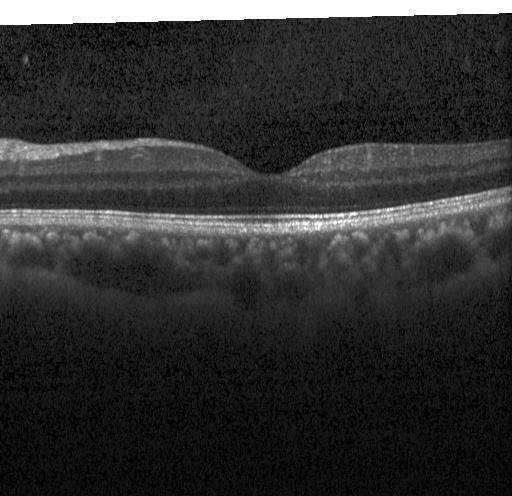

Spectral-domain optical coherence tomography · Heidelberg Spectralis OCT system · OCT line scan · fovea-centered — OCT finding: no choroidal neovascularization, no diabetic macular edema, and no drusen.